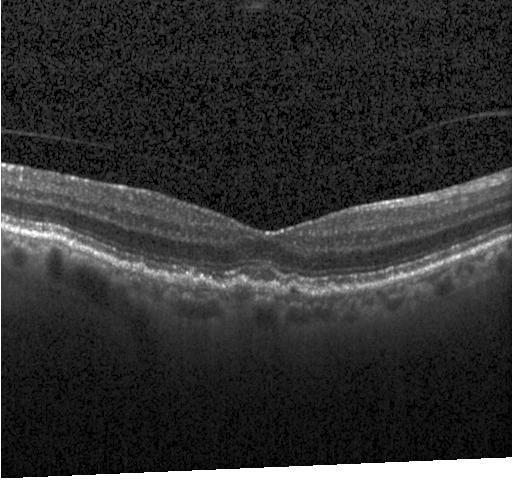 OCT B-scan showing sub-RPE drusenoid deposits.